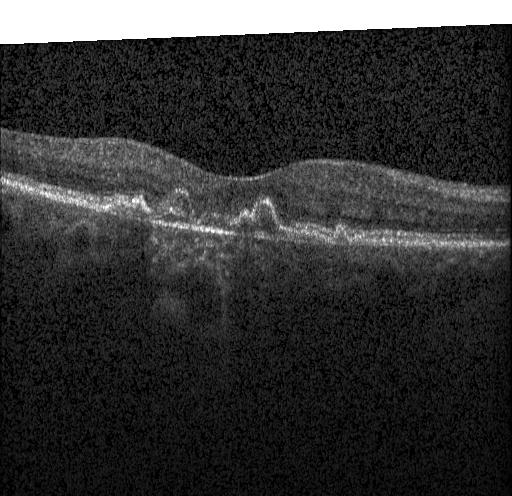

Finding: a choroidal neovascular membrane.